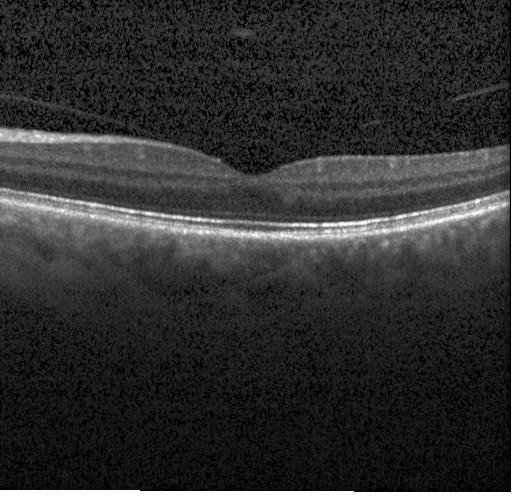
Retinal OCT cross-section. Finding: no choroidal neovascularization, no diabetic macular edema, and no drusen.